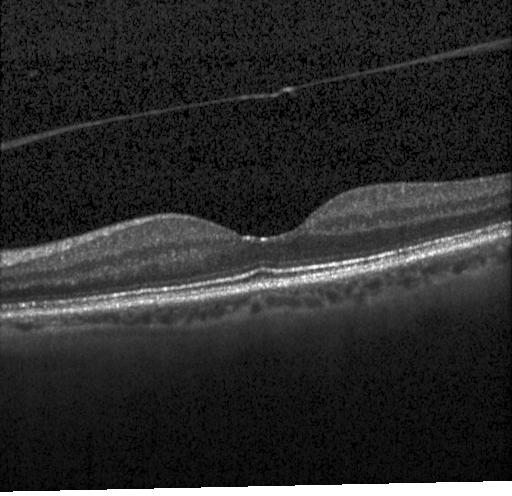

Heidelberg Spectralis, OCT line scan, through the macula.
Dx: no CNV, no DME, and no drusen.